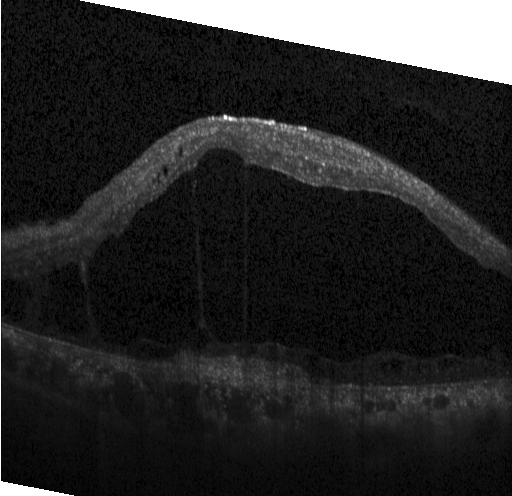
Spectral-domain OCT. Horizontal scan through the fovea. Optical coherence tomography scan. DME.